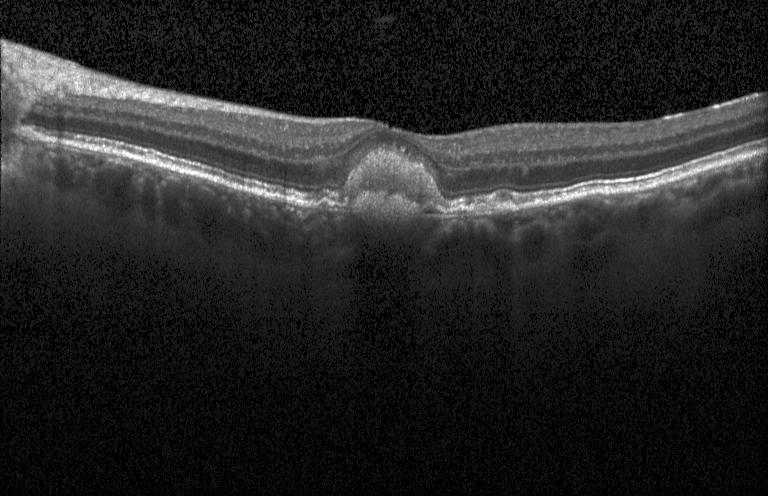 Through the macula. OCT line scan. Spectral-domain optical coherence tomography
OCT finding: CNV.